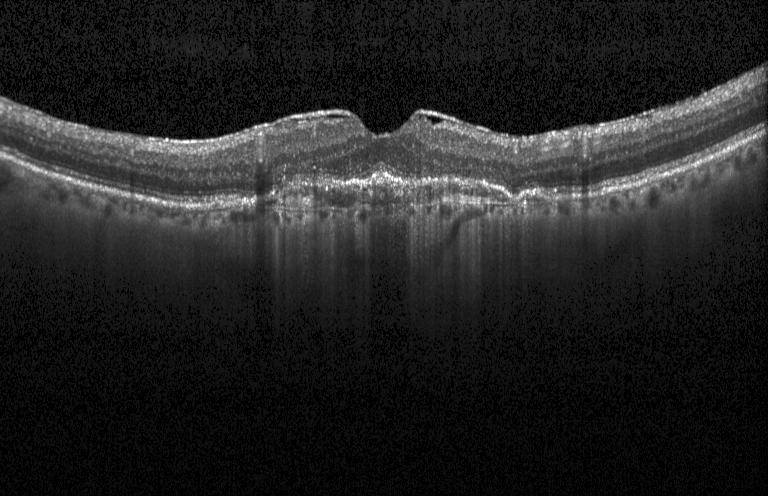
Heidelberg Spectralis. Spectral-domain OCT. Centered on the fovea. Optical coherence tomography B-scan — The scan shows CNV.